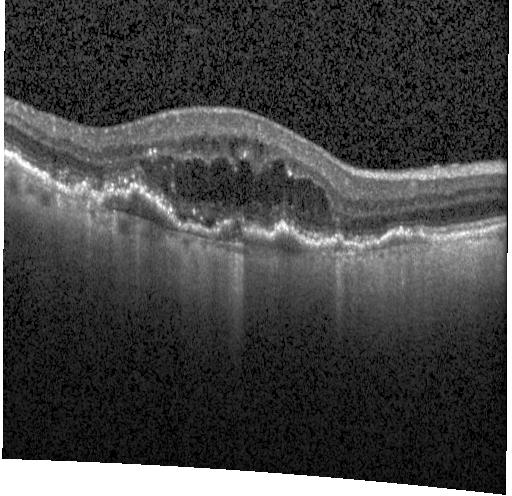 Acquired on a Heidelberg Spectralis · retinal OCT cross-section. Impression: a choroidal neovascular membrane.